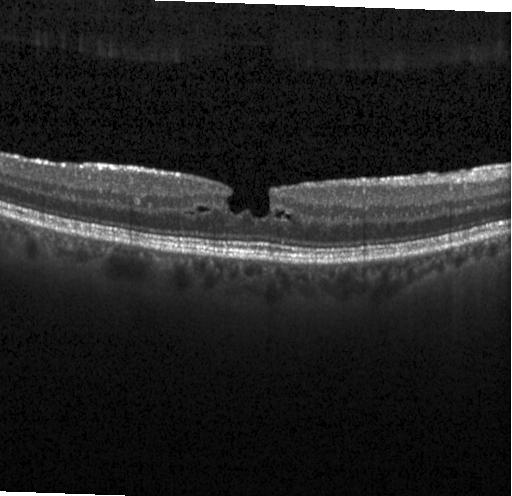 Retinal OCT B-scan. Macular scan. Acquired on a Heidelberg Spectralis. Spectral-domain OCT.
Assessment: diabetic macular edema (DME).